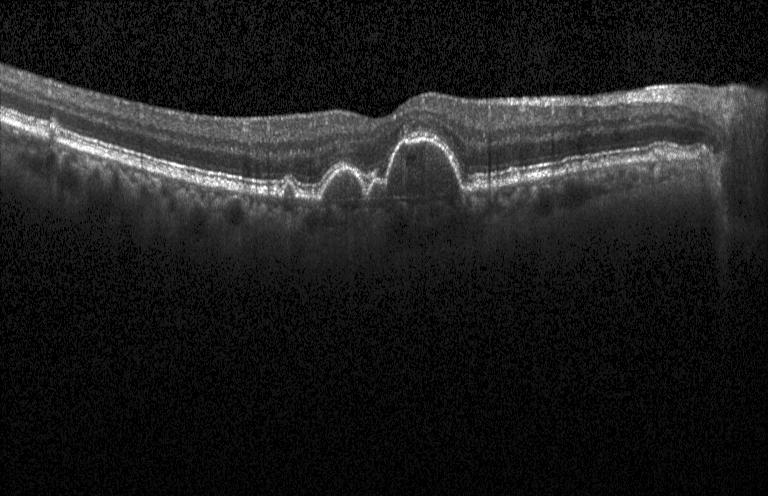
Optical coherence tomography scan, spectral-domain OCT
Impression: drusen.